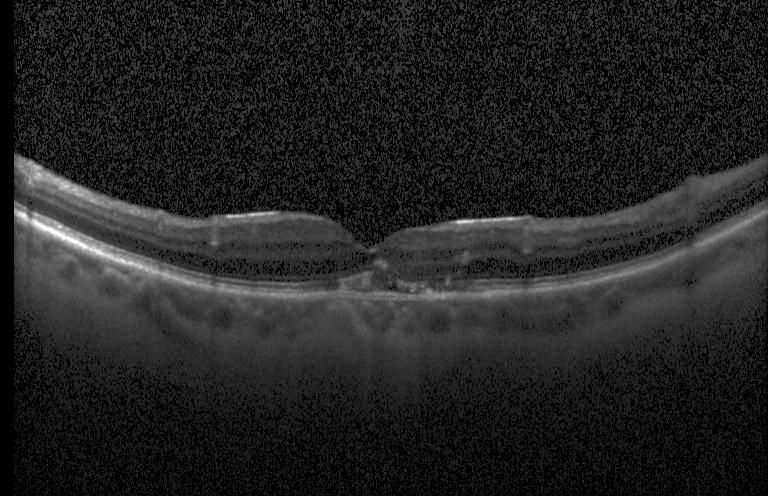
Finding: choroidal neovascularization (CNV).